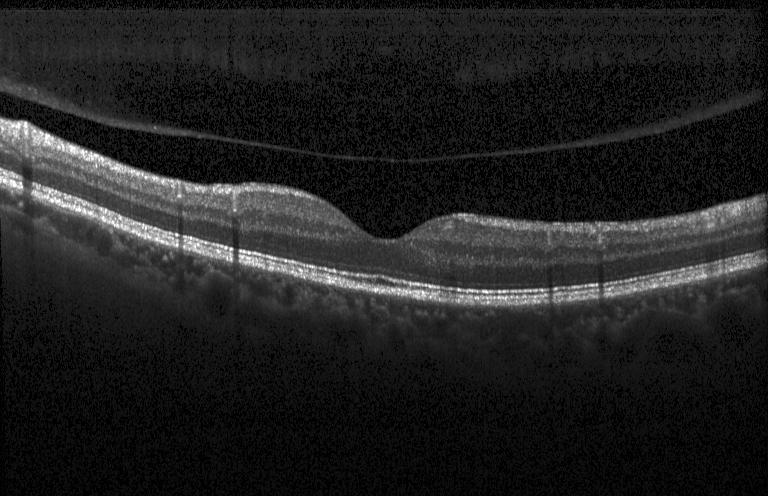
Optical coherence tomography B-scan · spectral-domain optical coherence tomography · instrument: Heidelberg Spectralis · macular scan. Assessment: no choroidal neovascularization, diabetic macular edema, or drusen.